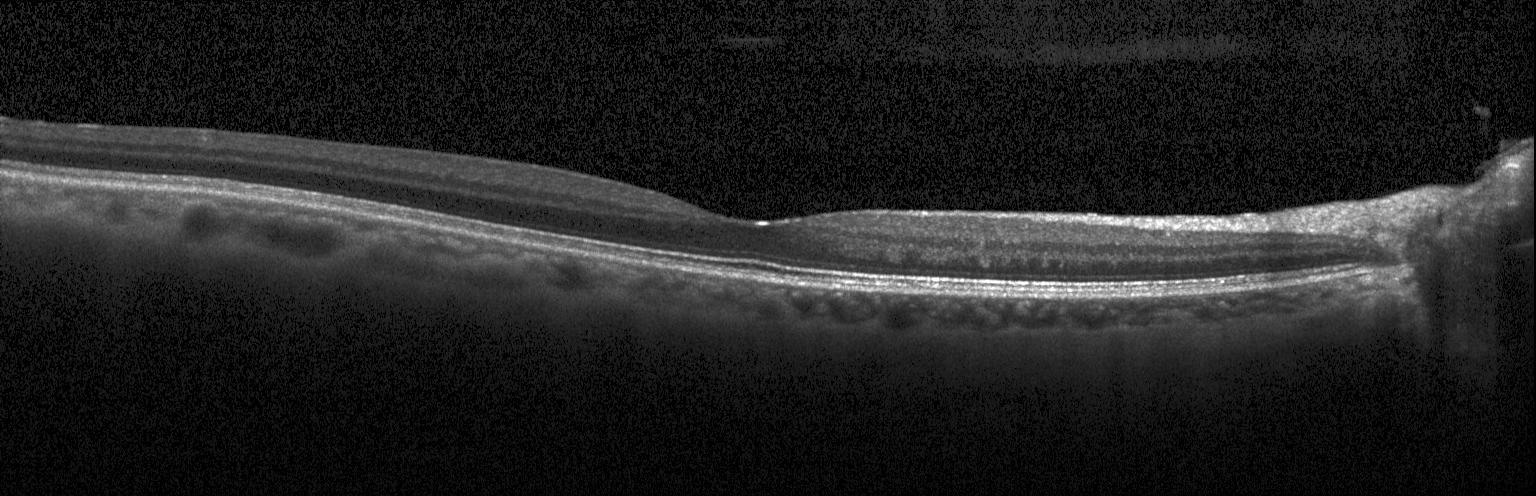

Centered on the fovea · acquired on a Heidelberg Spectralis · optical coherence tomography scan.
Finding: neither CNV, DME, nor drusen.